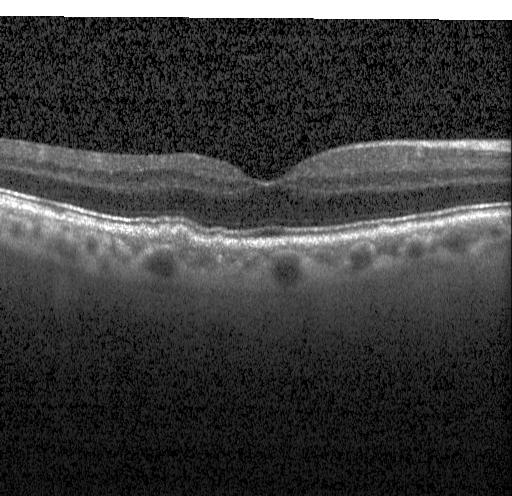 OCT B-scan.
This B-scan demonstrates sub-RPE drusenoid deposits.